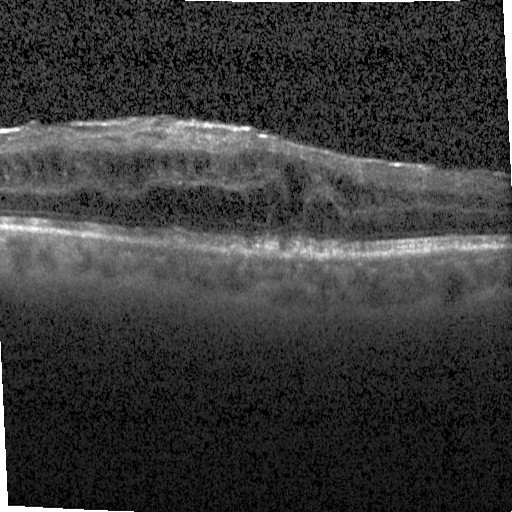
Diagnosis: DME.